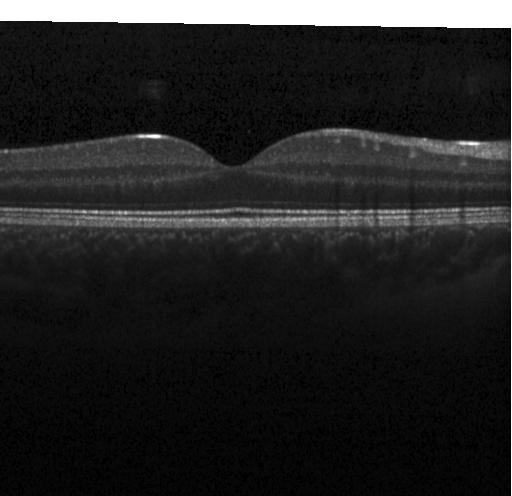 Fovea-centered. SD-OCT. OCT line scan. Instrument: Heidelberg Spectralis — Impression: no choroidal neovascularization, no diabetic macular edema, and no drusen.